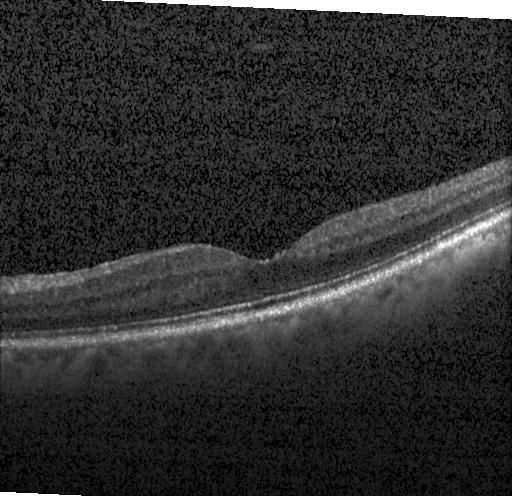
SD-OCT. Heidelberg Spectralis OCT system. Optical coherence tomography B-scan.
Neither choroidal neovascularization, diabetic macular edema, nor drusen.